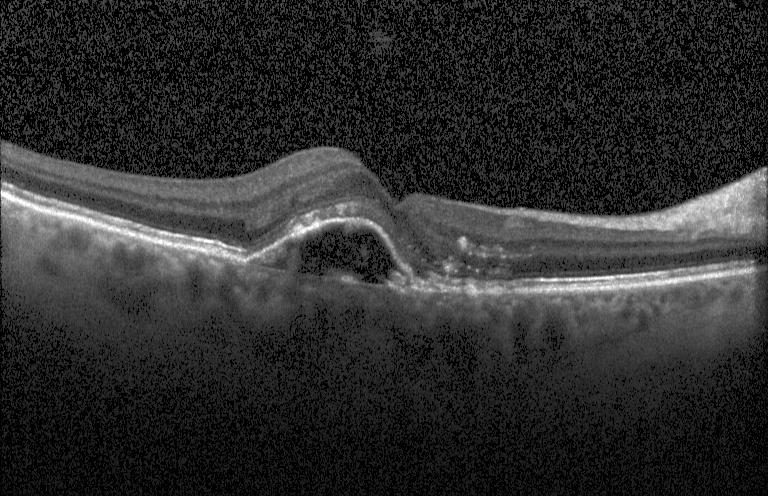 OCT finding: a choroidal neovascular membrane.